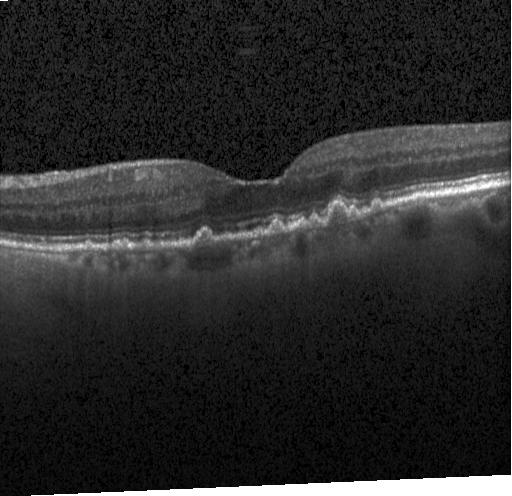
OCT scan showing multiple drusen.